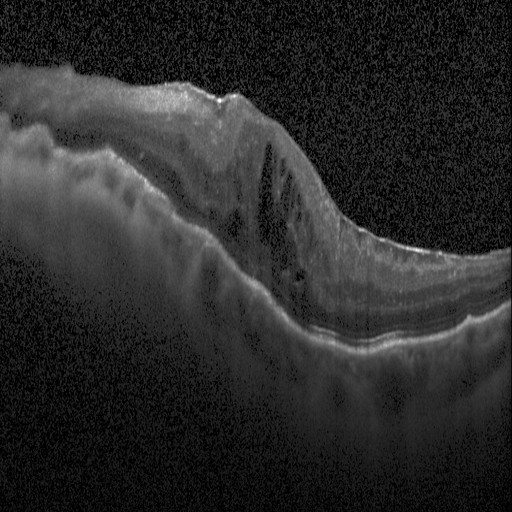
Assessment: diabetic macular edema.